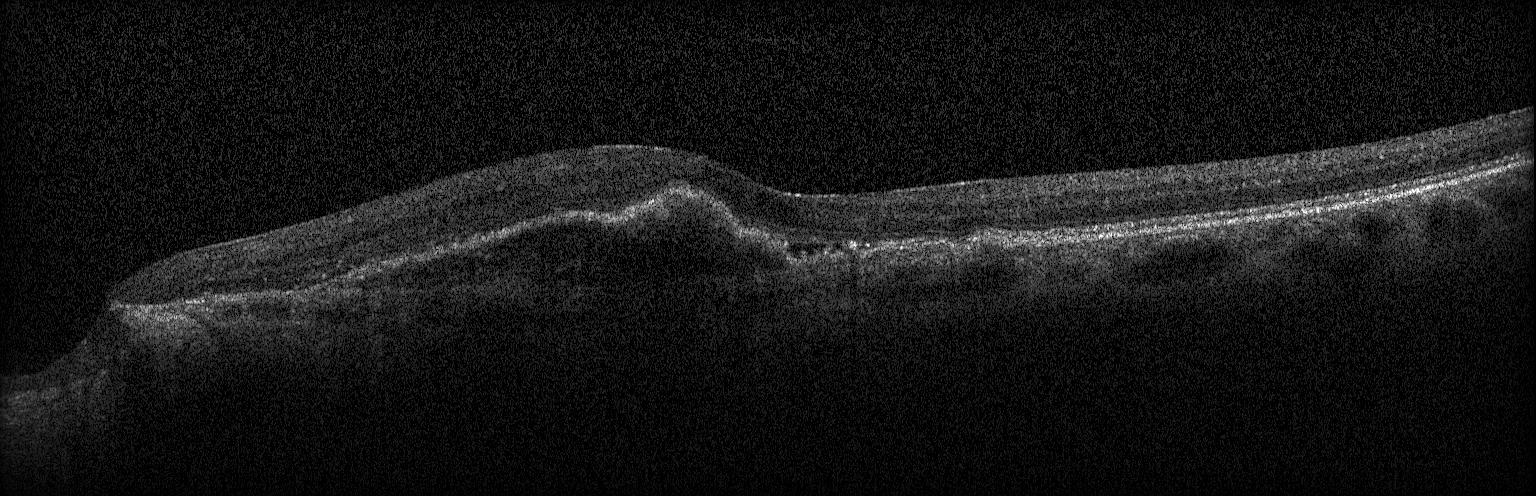

Dx: a choroidal neovascular membrane.